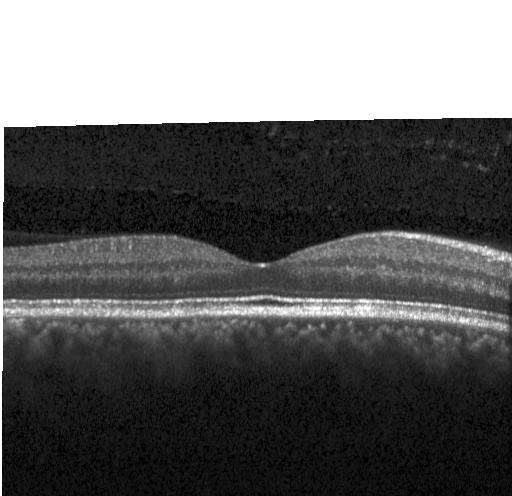 Finding: no evidence of choroidal neovascularization, diabetic macular edema, or drusen.